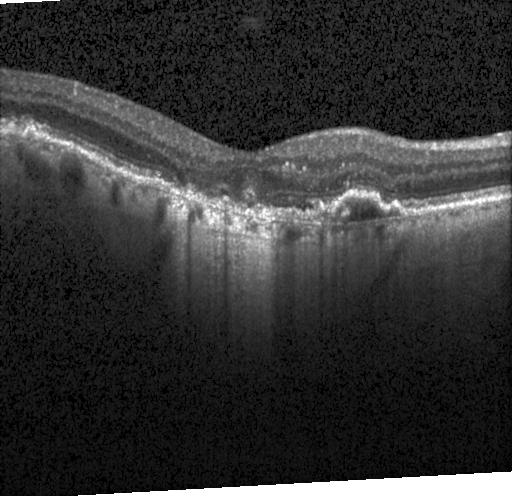 Macular OCT: a choroidal neovascular membrane.